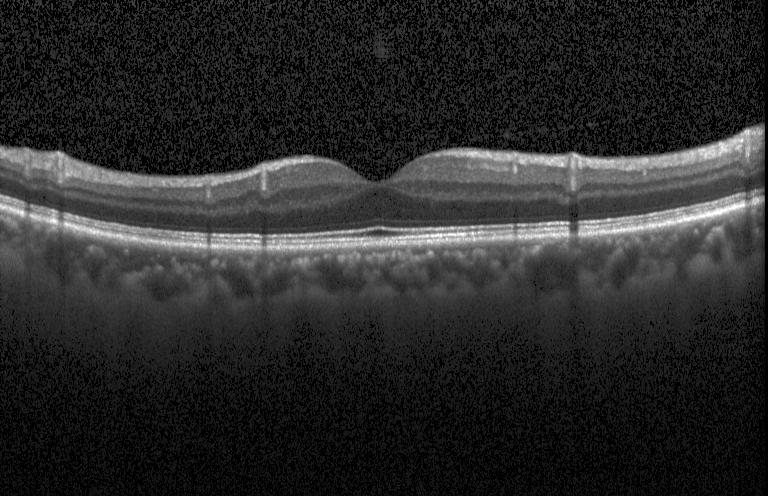

OCT B-scan; instrument: Heidelberg Spectralis; spectral-domain OCT; through the macula. Assessment: no CNV, DME, or drusen.